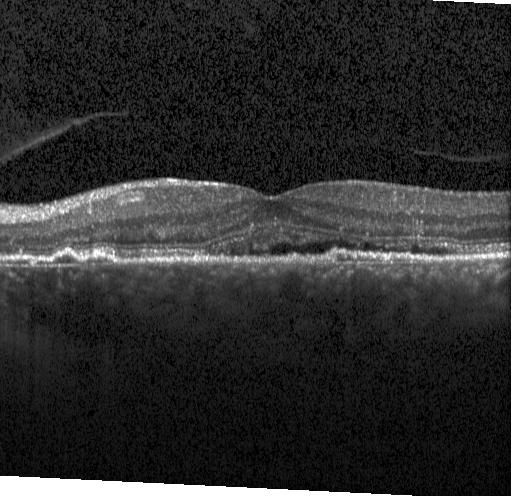 Spectral-domain optical coherence tomography, optical coherence tomography scan, Heidelberg Spectralis
Diagnosis: a choroidal neovascular membrane.